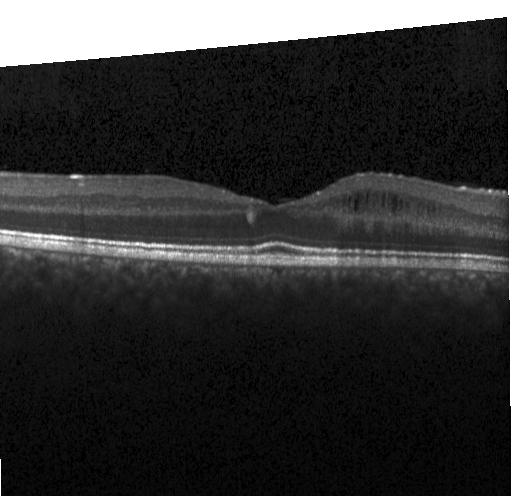 Heidelberg Spectralis · spectral-domain OCT · OCT B-scan.
Impression: DME.